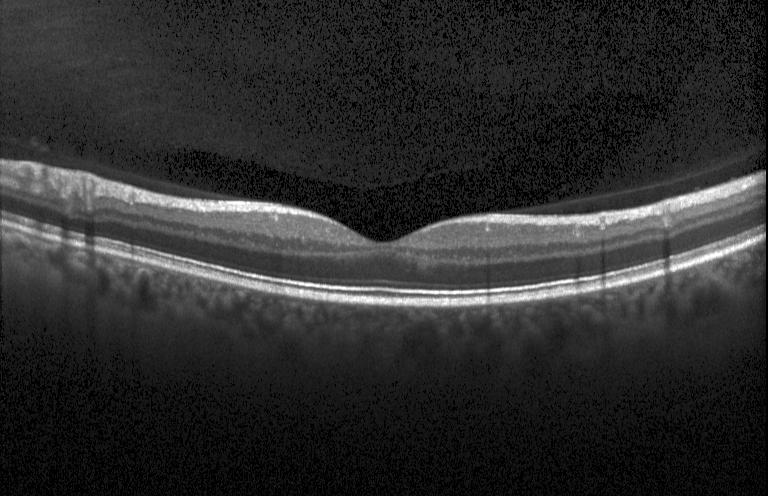

OCT finding: no CNV, DME, or drusen.